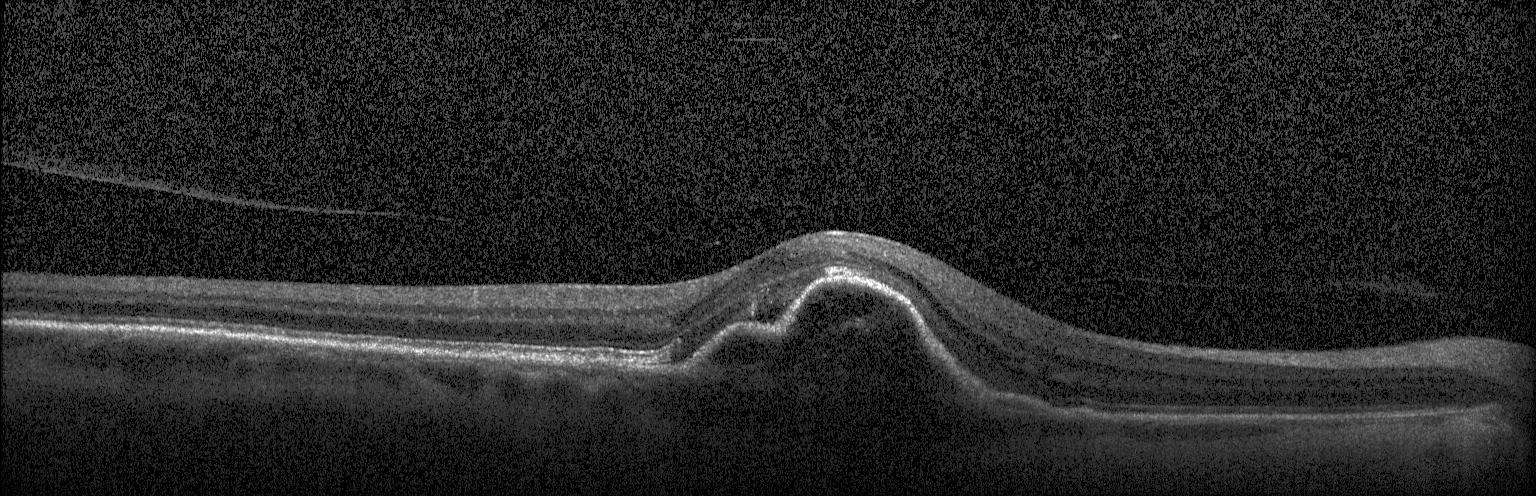 Optical coherence tomography B-scan · Heidelberg Spectralis · through the macula — Diagnosis: choroidal neovascularization.